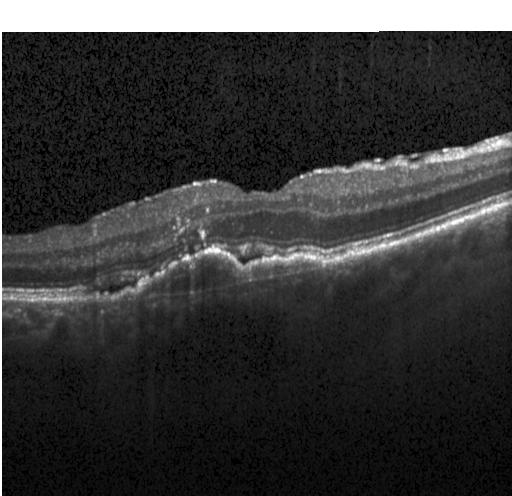

Dx: choroidal neovascularization.